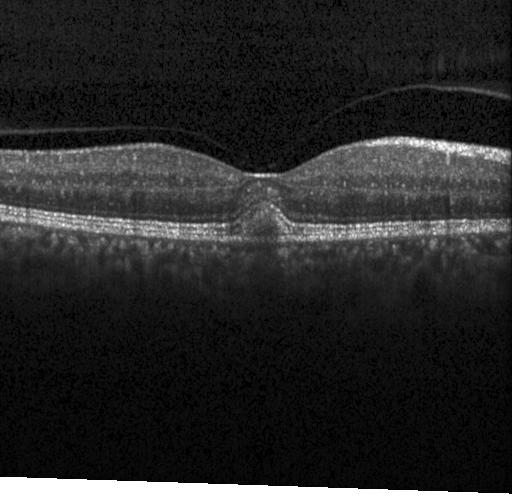

SD-OCT; OCT B-scan — Assessment: a choroidal neovascular membrane.